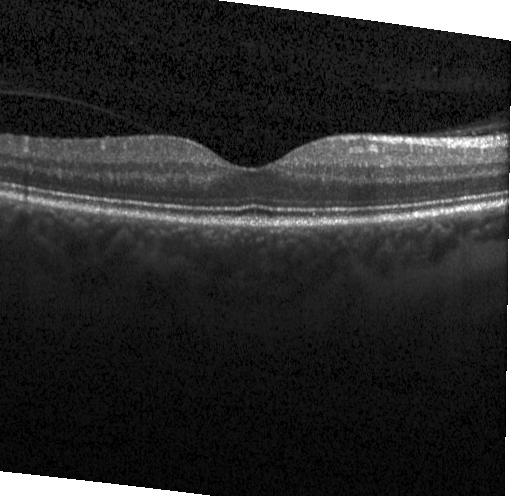

Diagnosis: neither CNV, DME, nor drusen.